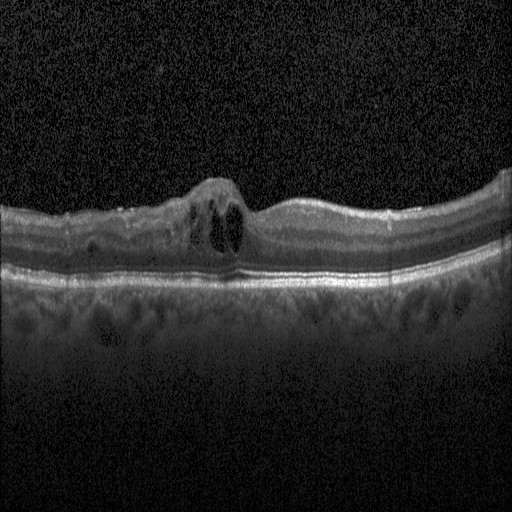 Diabetic macular edema.